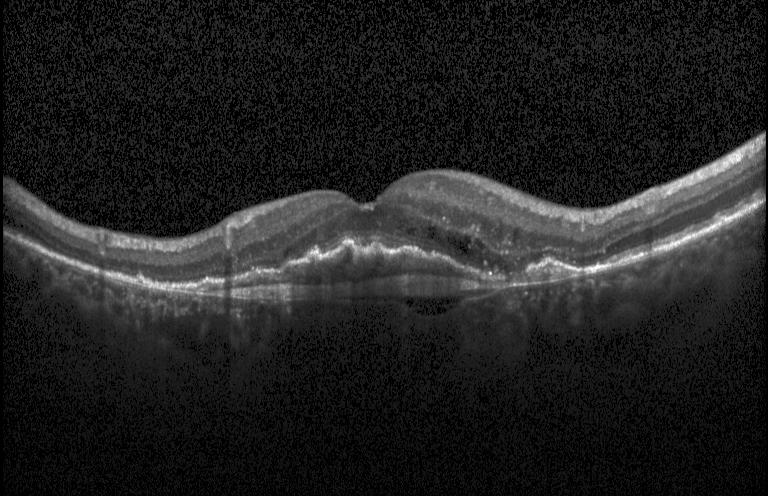 Spectral-domain OCT. OCT B-scan
The scan shows a choroidal neovascular membrane.